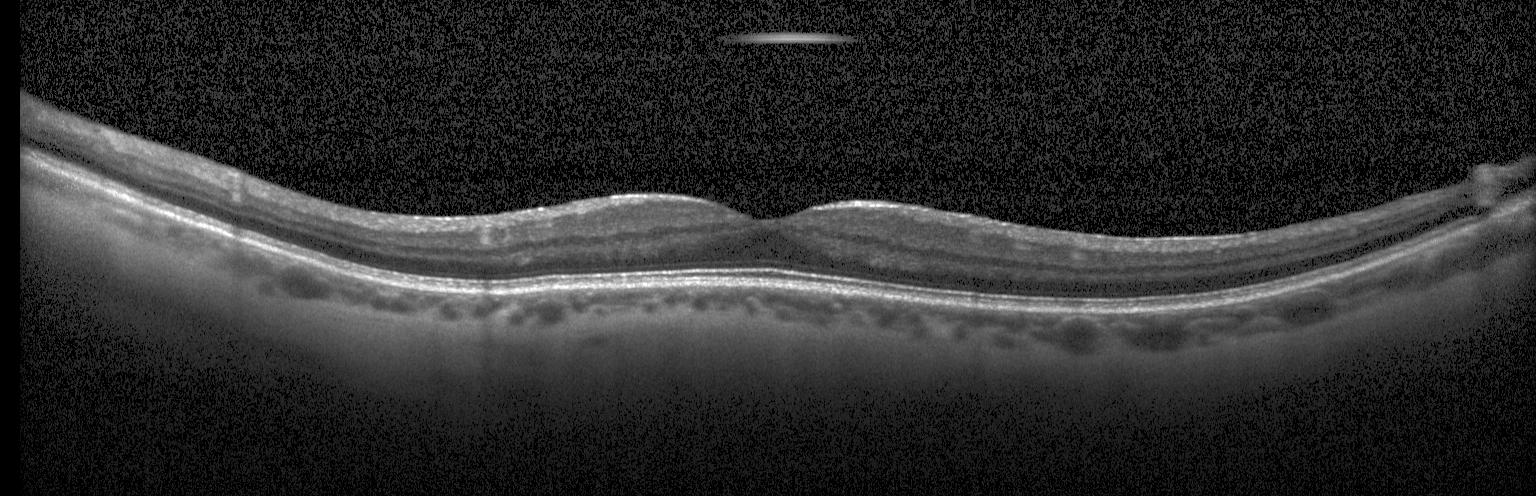 Impression: no CNV, no DME, and no drusen.